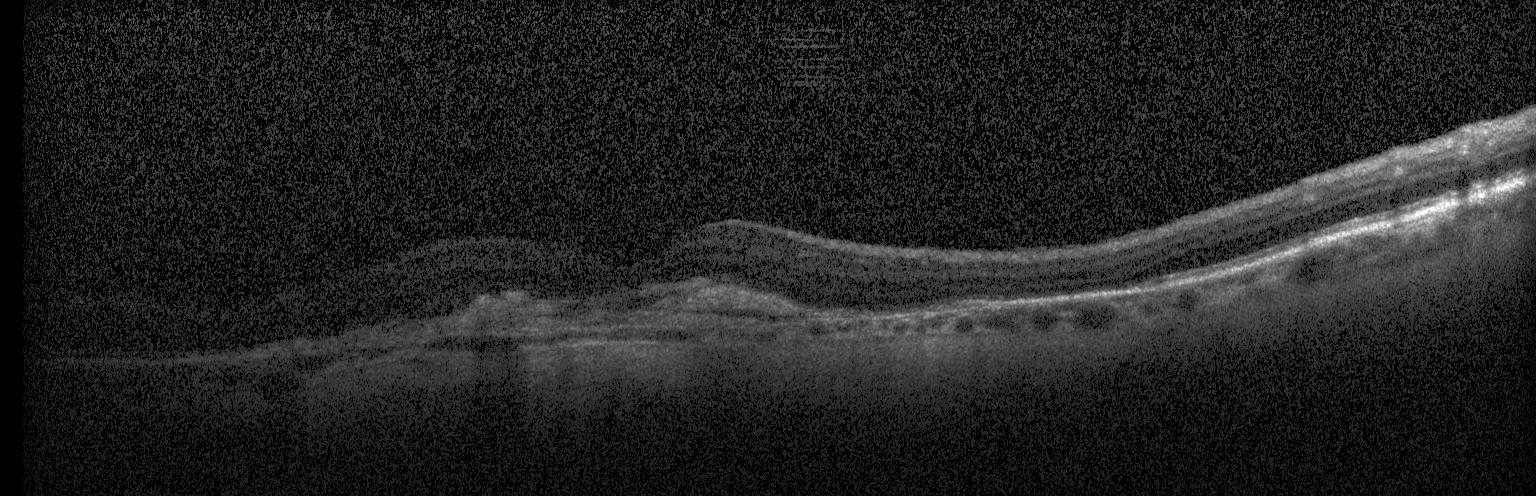 Dx: a choroidal neovascular membrane.